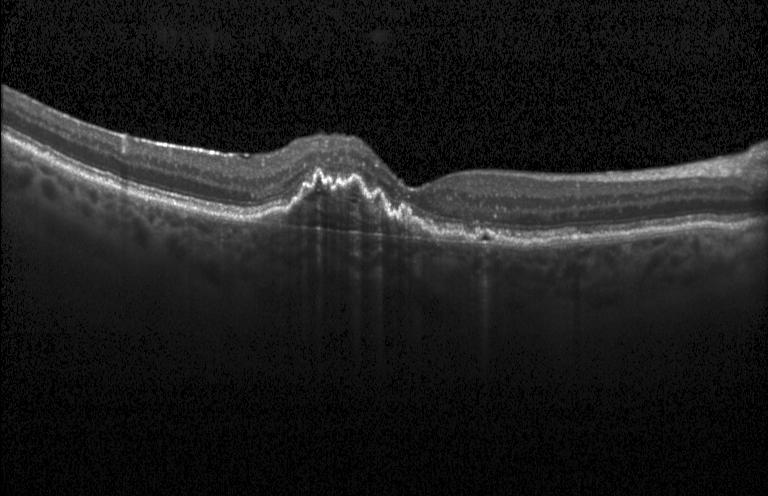

OCT line scan
Macular OCT: choroidal neovascularization.